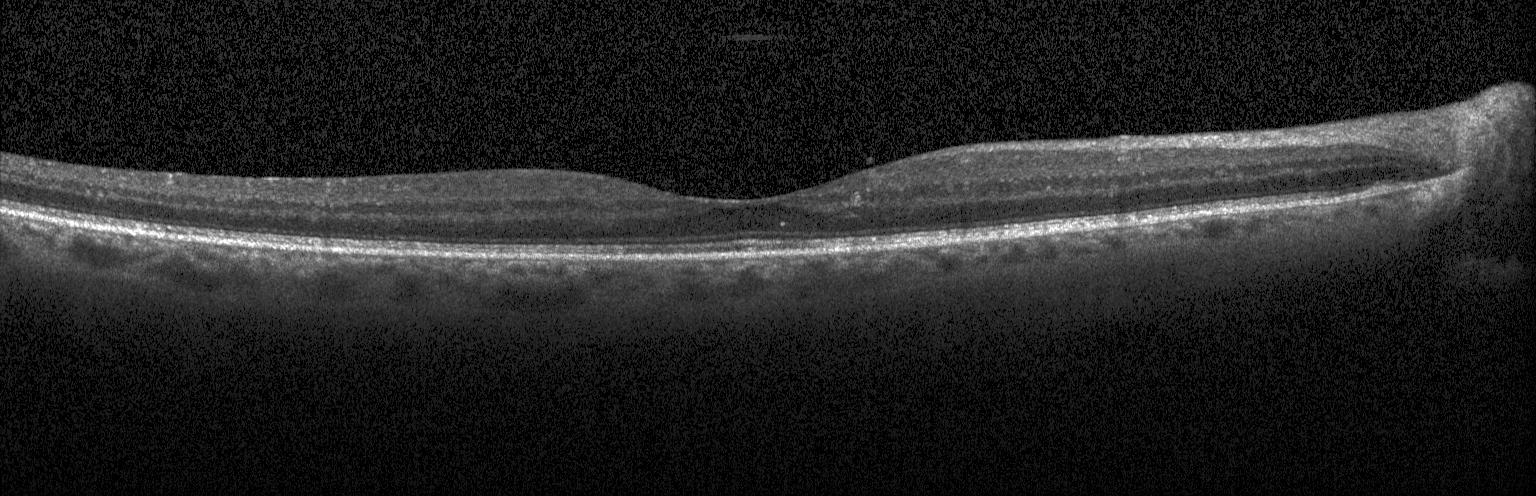 Finding: no evidence of choroidal neovascularization, diabetic macular edema, or drusen.